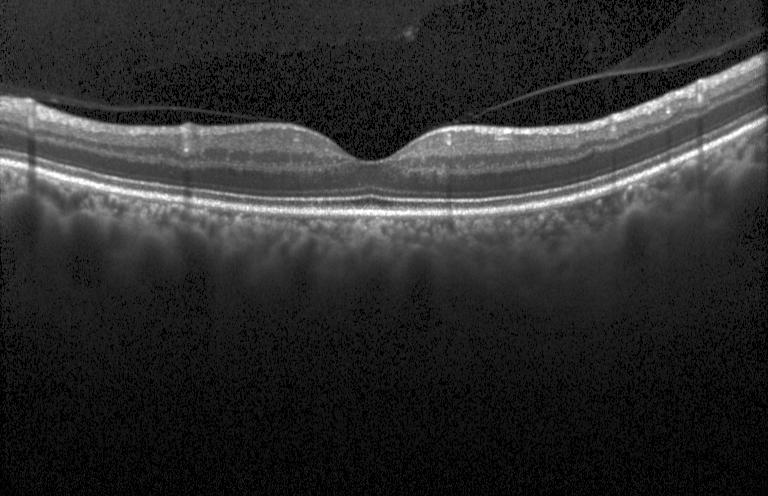
Spectral-domain OCT B-scan: no evidence of choroidal neovascularization, diabetic macular edema, or drusen.